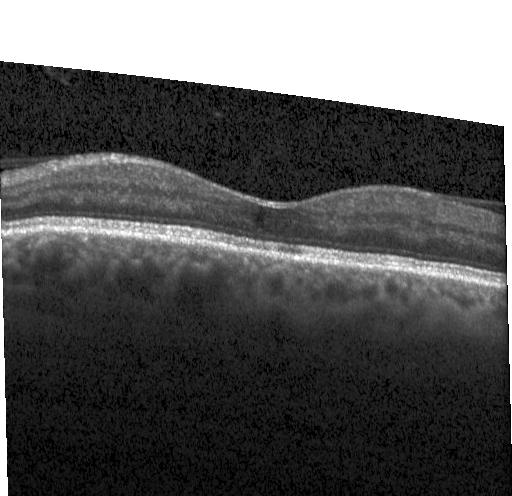
OCT B-scan; Heidelberg Spectralis; spectral-domain OCT — The scan shows no CNV, DME, or drusen.